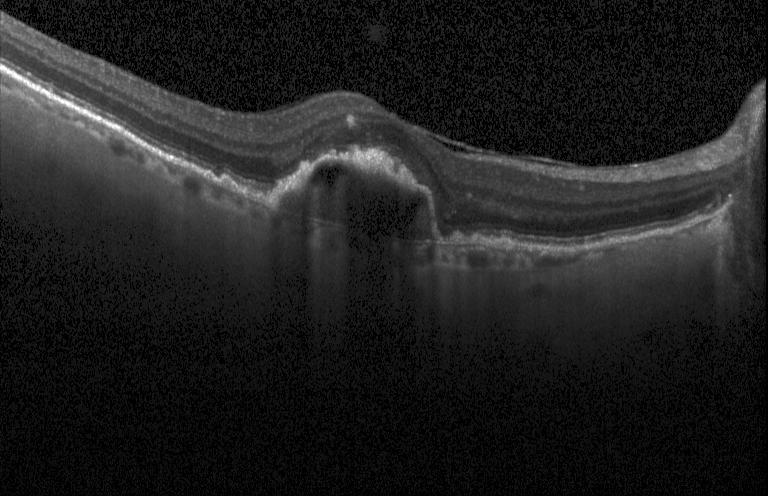
Instrument: Heidelberg Spectralis, retinal OCT B-scan, fovea-centered
Diagnosis: a choroidal neovascular membrane.